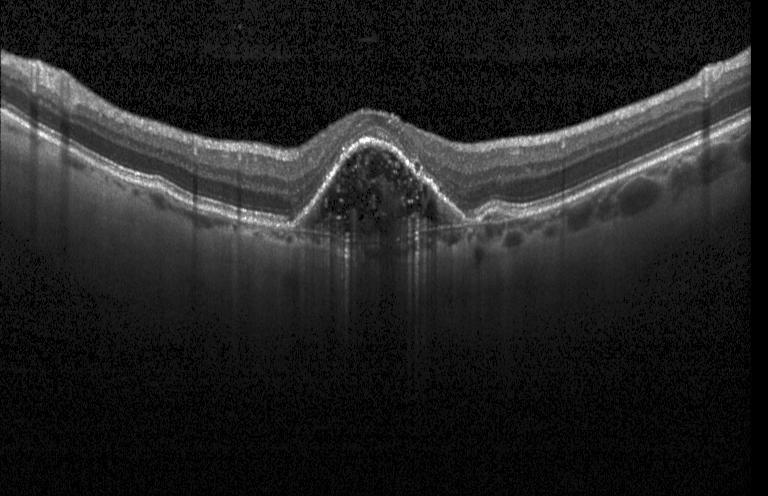
Horizontal scan through the fovea. Heidelberg Spectralis OCT system. Optical coherence tomography scan. Spectral-domain OCT
Assessment: a choroidal neovascular membrane.